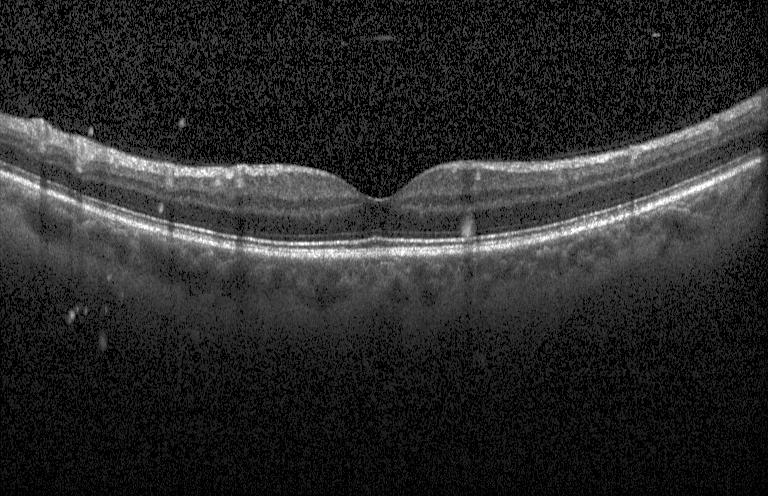 Retinal OCT cross-section · Heidelberg Spectralis · macular scan · SD-OCT. Diagnosis: no evidence of choroidal neovascularization, diabetic macular edema, or drusen.